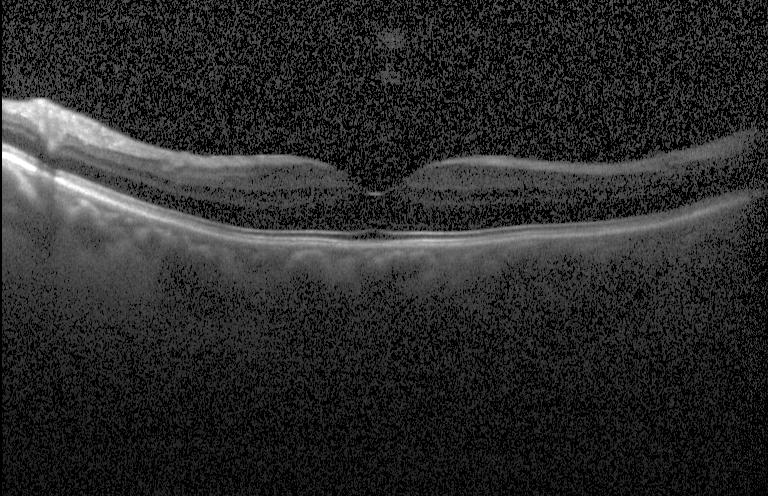

Heidelberg Spectralis · optical coherence tomography scan · fovea-centered.
Neither CNV, DME, nor drusen.